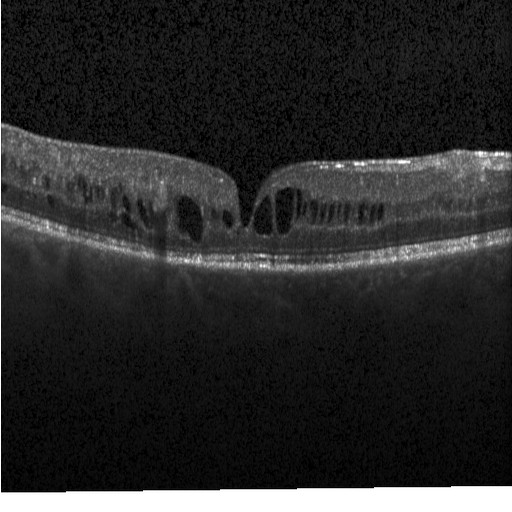 Spectral-domain OCT, OCT line scan, Heidelberg Spectralis, centered on the fovea — DME.